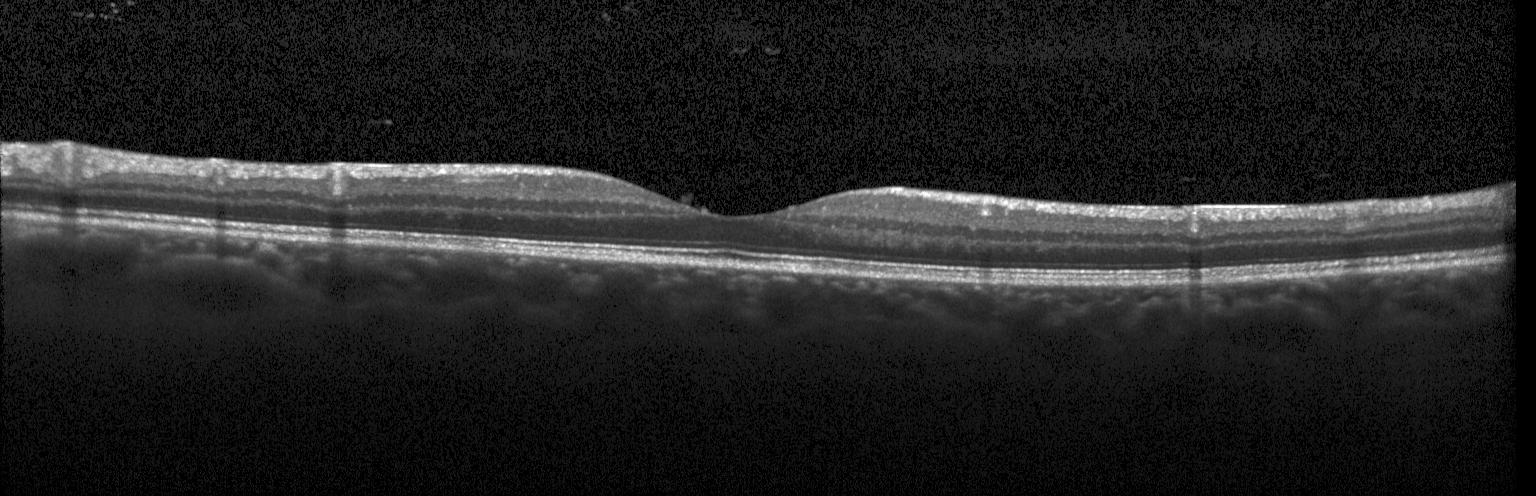 Optical coherence tomography scan
Finding: no CNV, DME, or drusen.